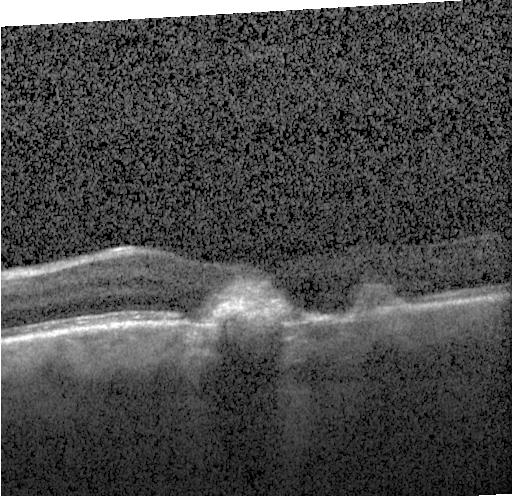 Optical coherence tomography scan. Instrument: Heidelberg Spectralis
Impression: choroidal neovascularization (CNV).